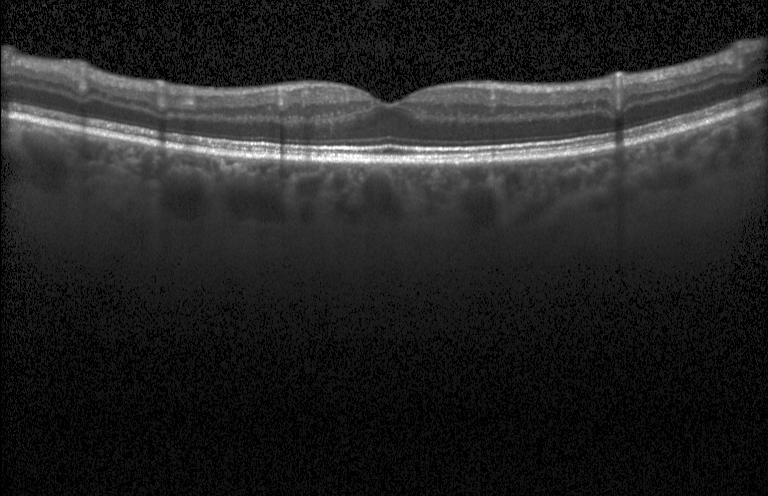
Optical coherence tomography B-scan, horizontal scan through the fovea.
Diagnosis: no evidence of CNV, DME, or drusen.